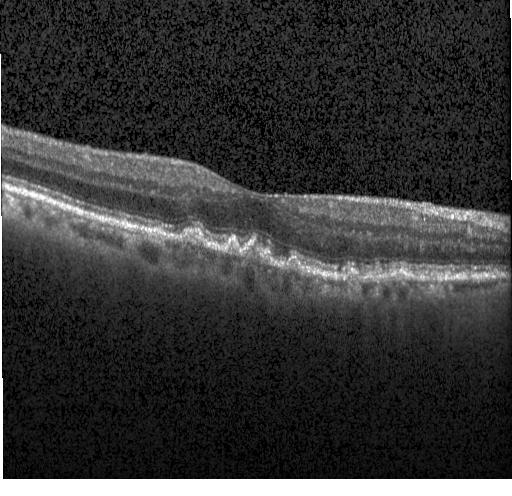
Heidelberg Spectralis · horizontal scan through the fovea · retinal OCT B-scan · SD-OCT — Impression: drusen.